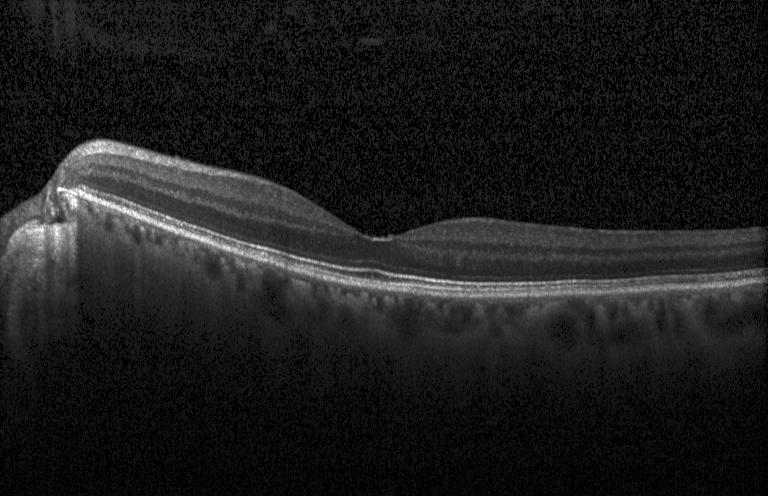 Macular scan. Acquired on a Heidelberg Spectralis. OCT line scan. Spectral-domain optical coherence tomography.
Assessment: no evidence of CNV, DME, or drusen.